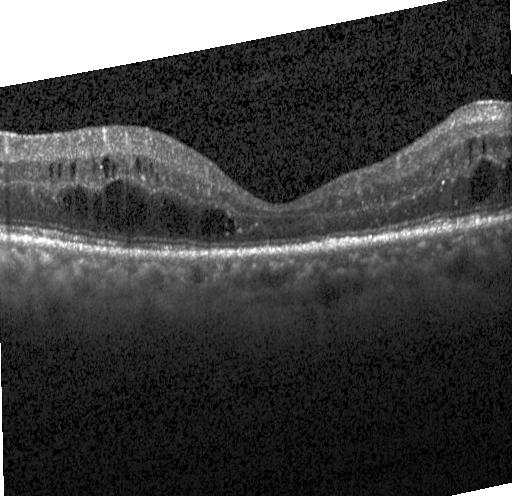

OCT line scan · through the macula · spectral-domain OCT.
Finding: diabetic macular edema.